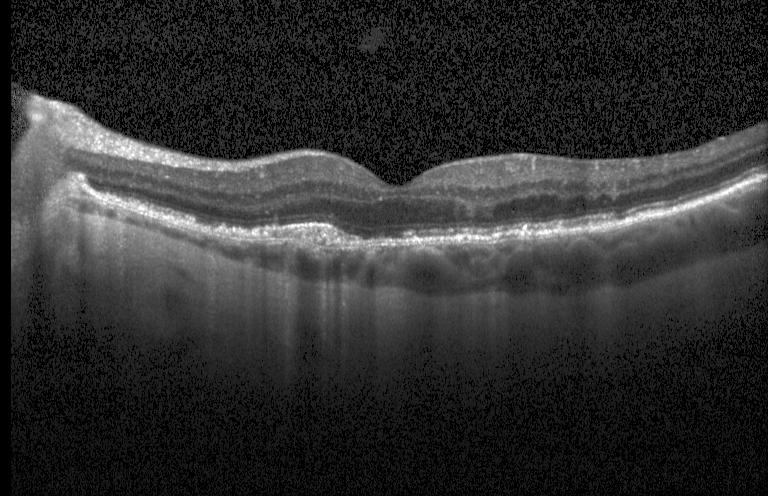

Retinal OCT cross-section
Impression: a choroidal neovascular membrane.